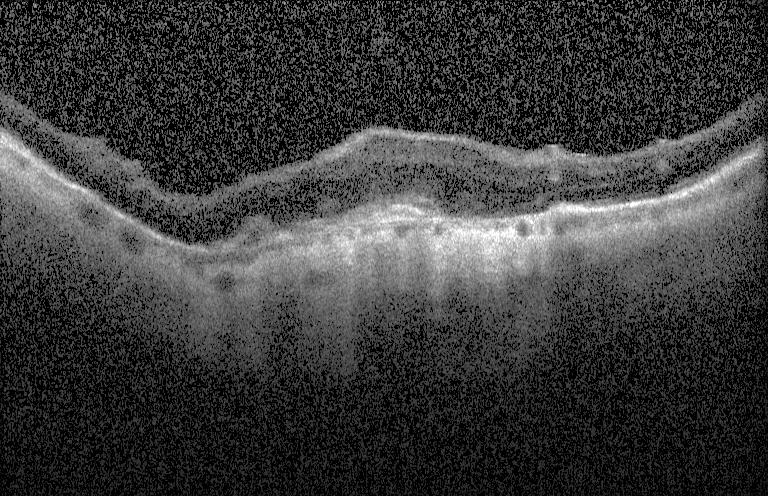 Finding: a choroidal neovascular membrane.